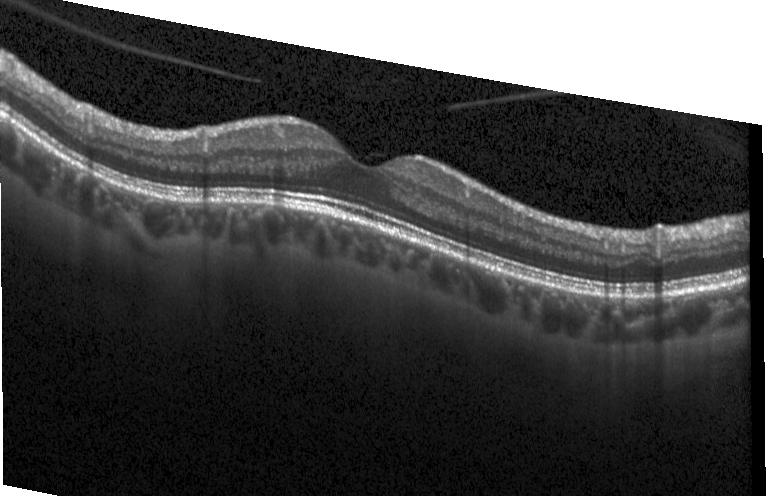

OCT scan showing no choroidal neovascularization, no diabetic macular edema, and no drusen.